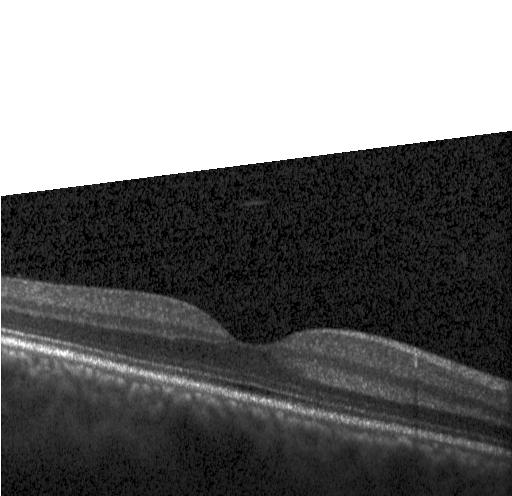
Acquired on a Heidelberg Spectralis; through the macula; spectral-domain optical coherence tomography; retinal OCT cross-section
Impression: no choroidal neovascularization, no diabetic macular edema, and no drusen.